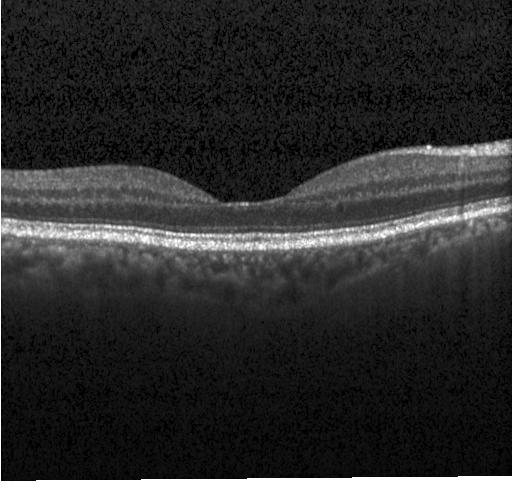
Retinal OCT cross-section showing neither choroidal neovascularization, diabetic macular edema, nor drusen.